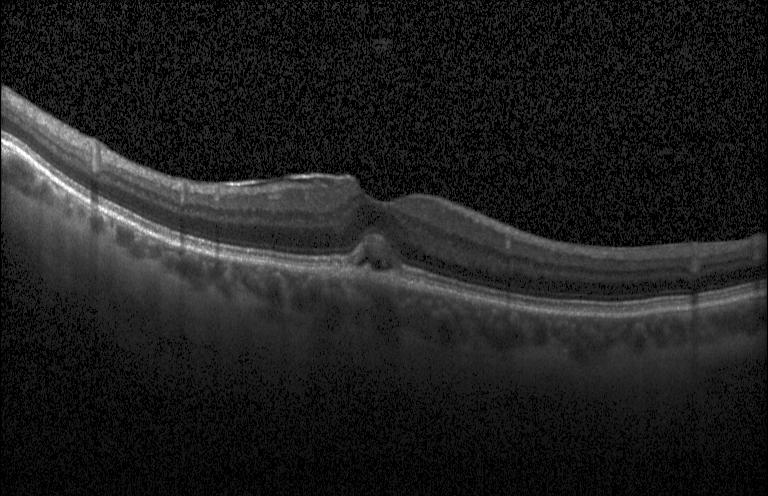 OCT scan showing choroidal neovascularization (CNV).